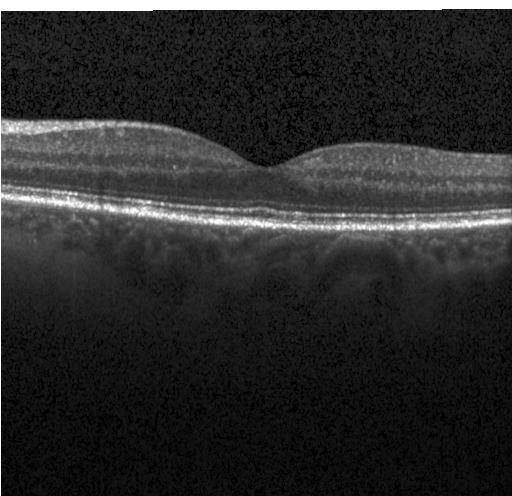 Spectral-domain OCT B-scan: neither choroidal neovascularization, diabetic macular edema, nor drusen.